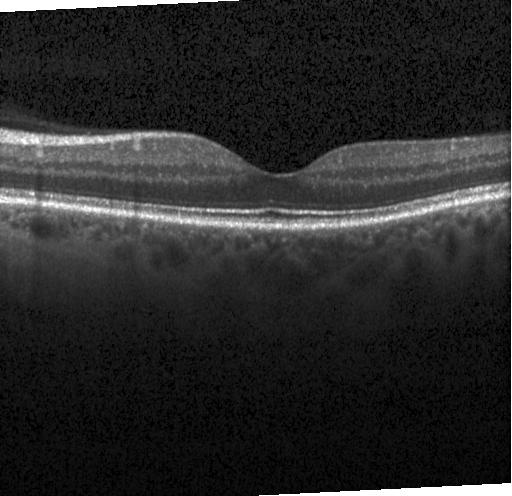
Macular scan · optical coherence tomography scan.
Macular OCT: no evidence of choroidal neovascularization, diabetic macular edema, or drusen.